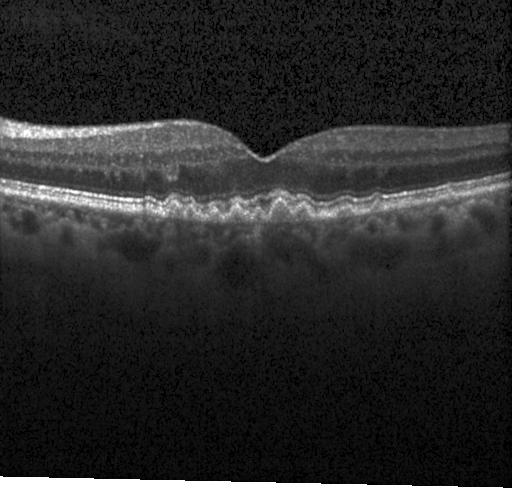

Impression: sub-RPE drusenoid deposits.